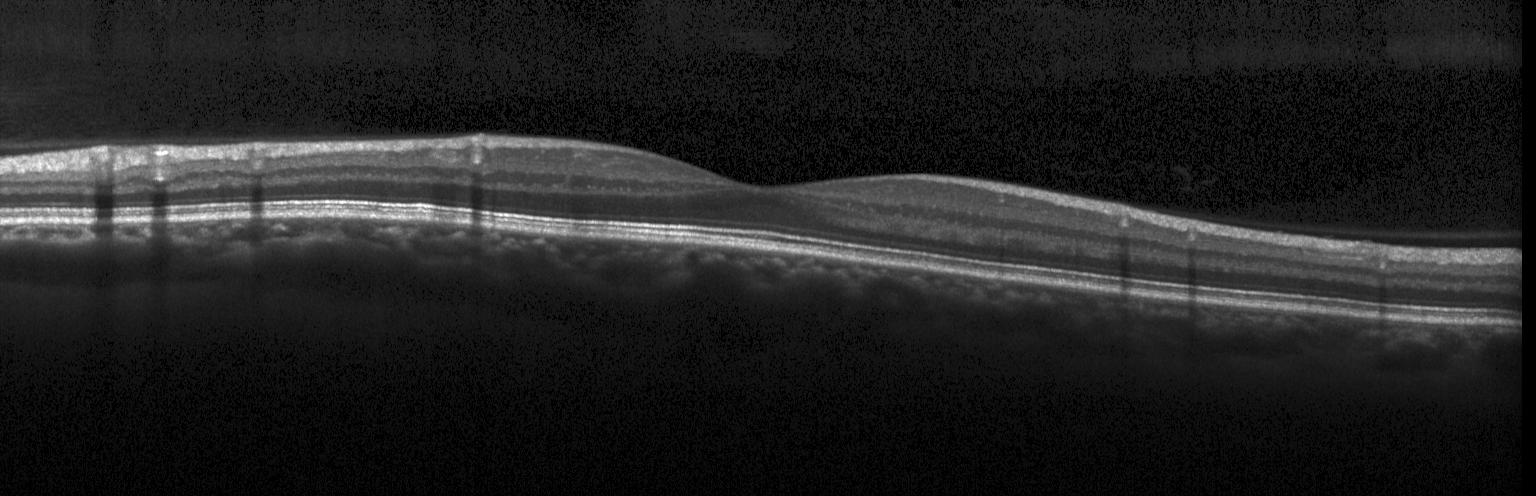 Optical coherence tomography B-scan. Macular OCT: no choroidal neovascularization, no diabetic macular edema, and no drusen.